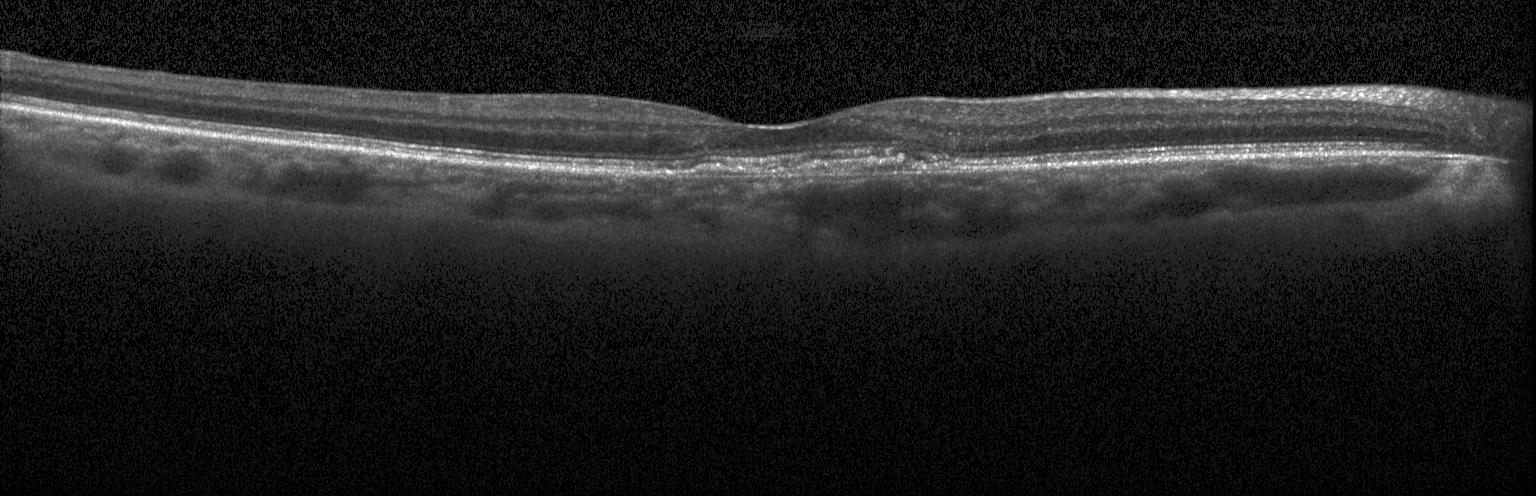
The scan shows a choroidal neovascular membrane.